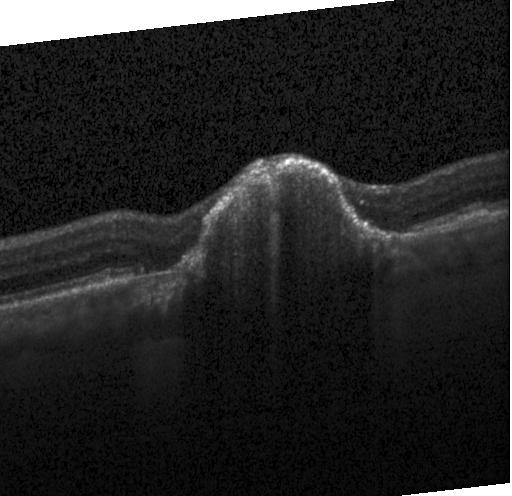
Retinal OCT cross-section showing CNV.